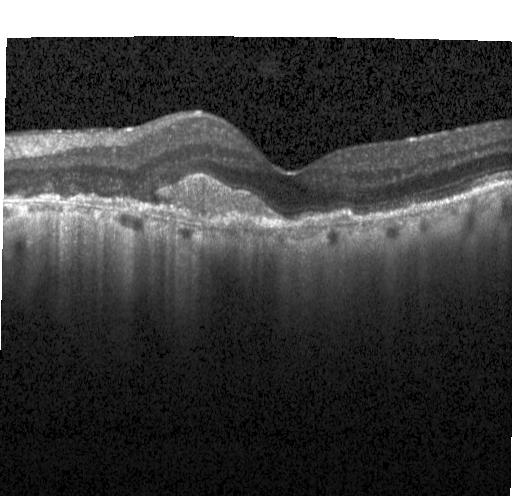 Retinal OCT cross-section; instrument: Heidelberg Spectralis — OCT finding: a choroidal neovascular membrane.